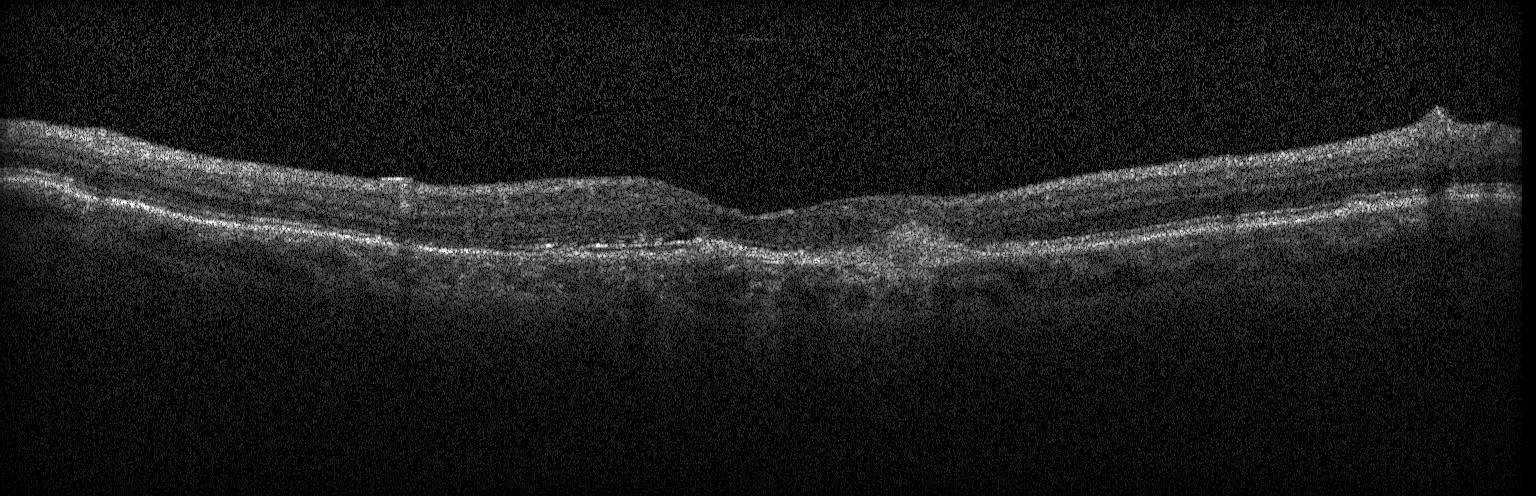

Instrument: Heidelberg Spectralis; fovea-centered; retinal OCT B-scan.
This B-scan demonstrates CNV.